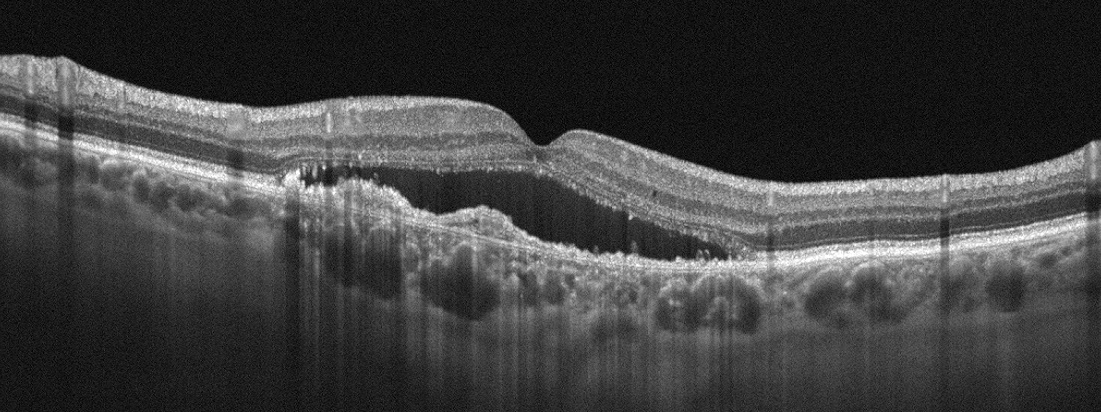
Fovea-centered · optical coherence tomography scan · acquired on an Optovue Avanti RTVue XR. OCT finding: age-related macular degeneration.